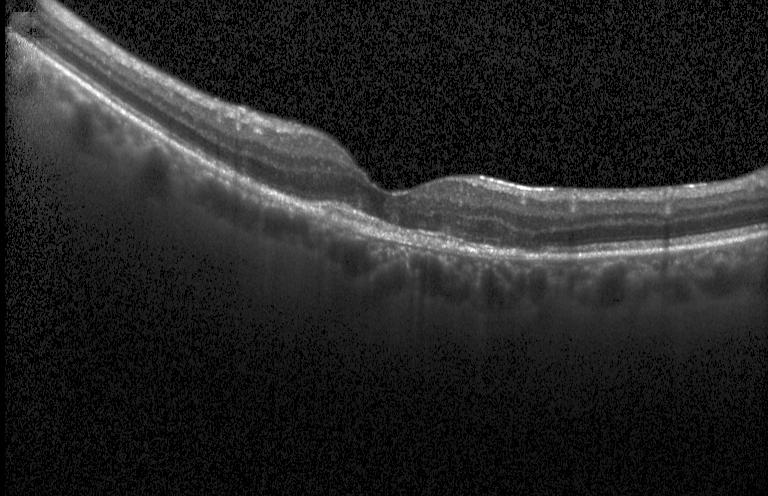 Acquired on a Heidelberg Spectralis · OCT line scan. Assessment: a choroidal neovascular membrane.